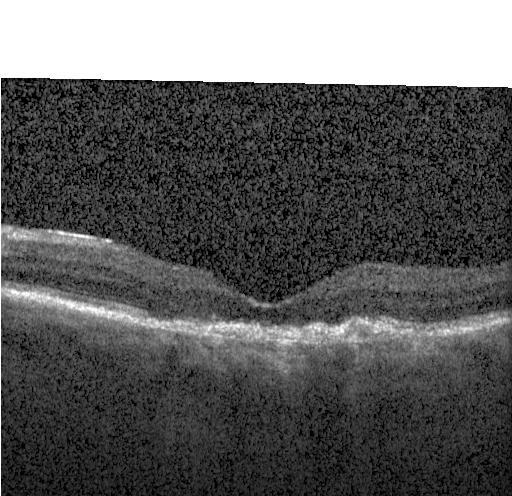 Optical coherence tomography B-scan, Heidelberg Spectralis — Diagnosis: a choroidal neovascular membrane.